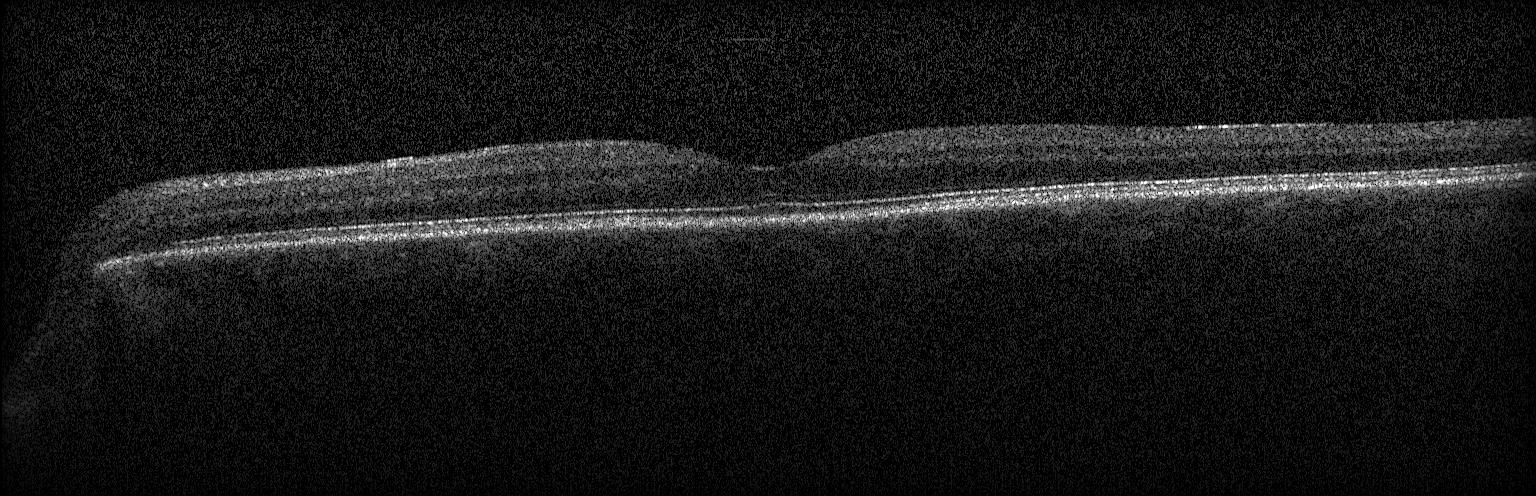

Heidelberg Spectralis; horizontal scan through the fovea; optical coherence tomography scan. Diagnosis: no evidence of CNV, DME, or drusen.